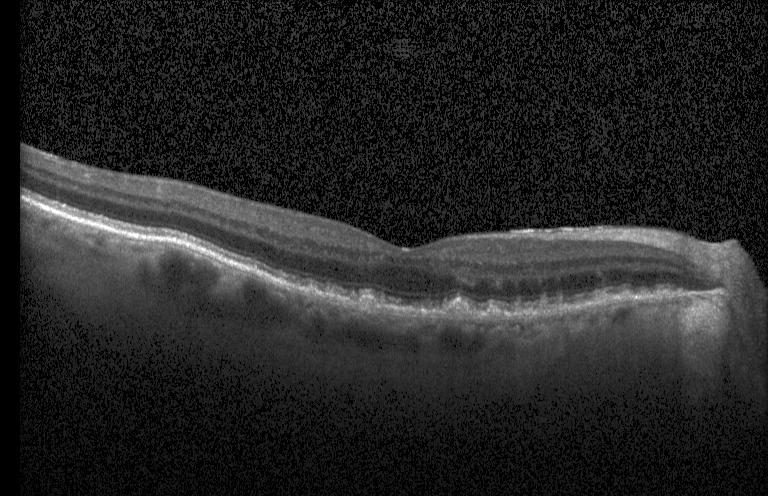
Retinal OCT B-scan. Diagnosis: drusen.